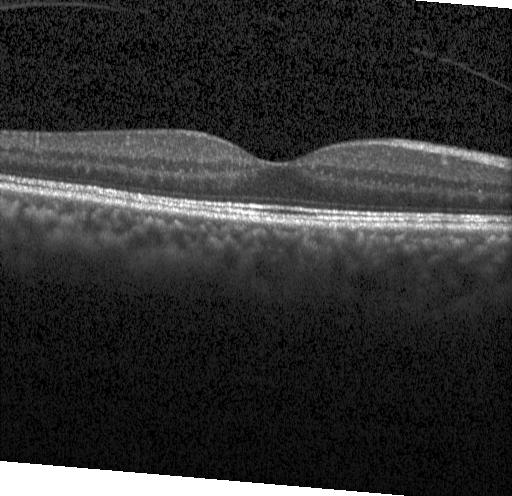
SD-OCT, macular scan, OCT B-scan.
No choroidal neovascularization, no diabetic macular edema, and no drusen.